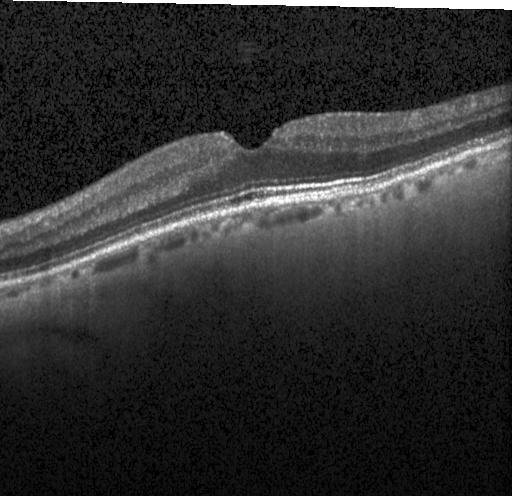 Horizontal scan through the fovea, spectral-domain optical coherence tomography, optical coherence tomography scan. Diagnosis: no evidence of CNV, DME, or drusen.